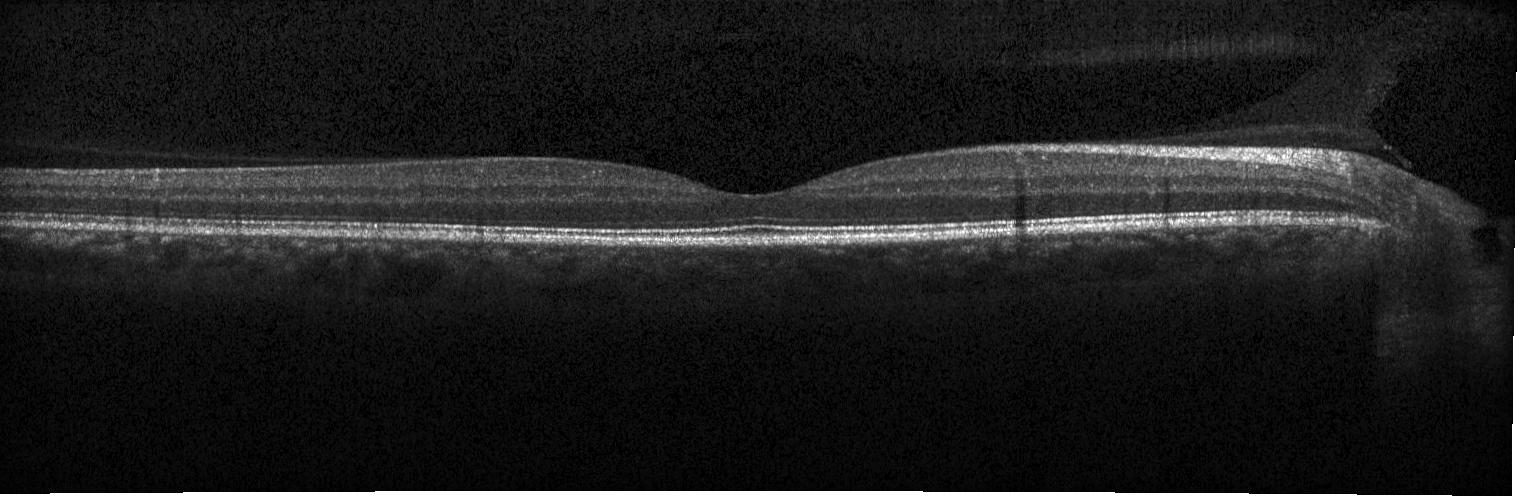 Diagnosis: no choroidal neovascularization, diabetic macular edema, or drusen.